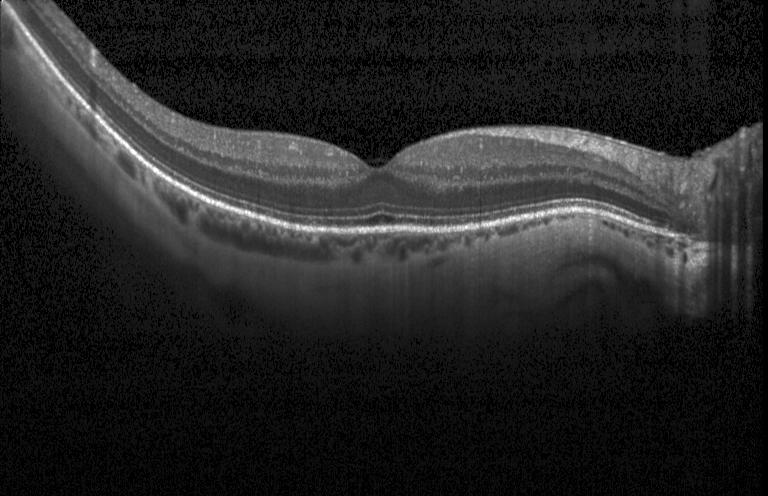 Dx: no choroidal neovascularization, diabetic macular edema, or drusen.